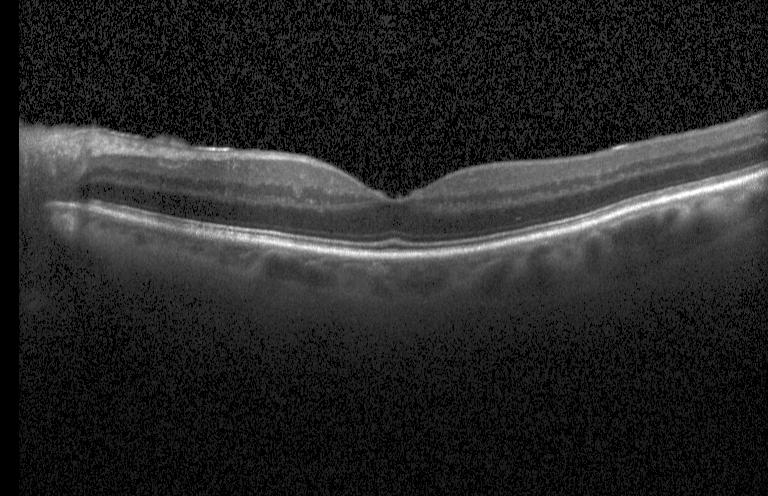

Finding: neither choroidal neovascularization, diabetic macular edema, nor drusen.